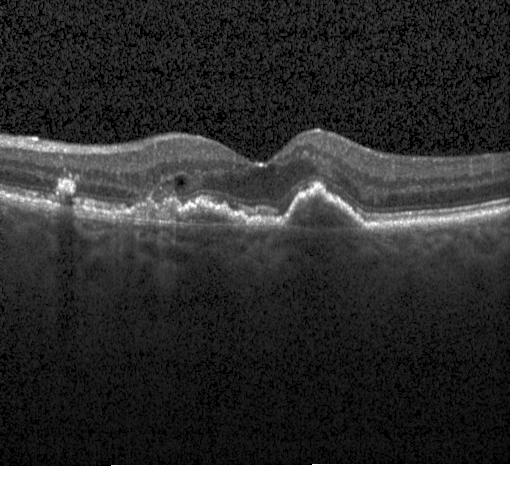
Spectral-domain OCT B-scan: a choroidal neovascular membrane.